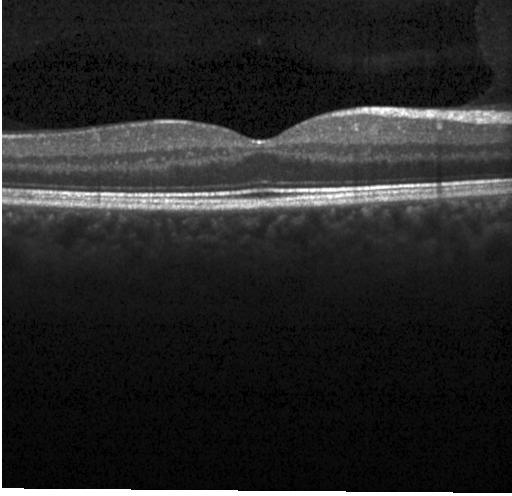

This B-scan demonstrates no evidence of CNV, DME, or drusen.